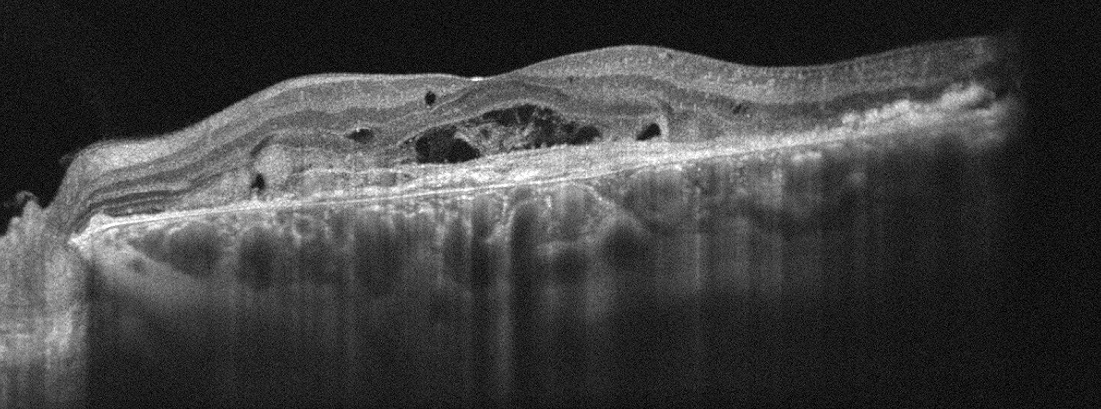

OCT finding: age-related macular degeneration.